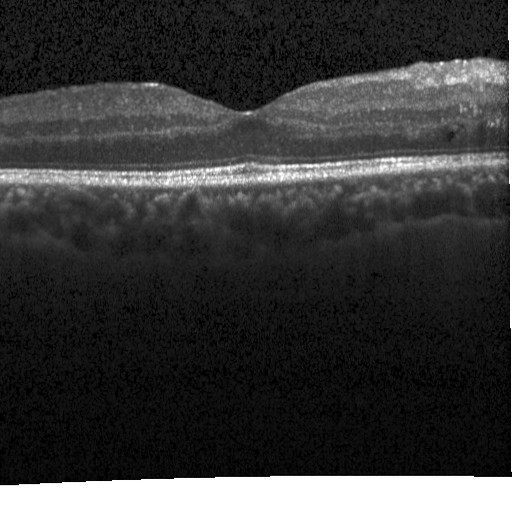 Diabetic macular edema (DME).